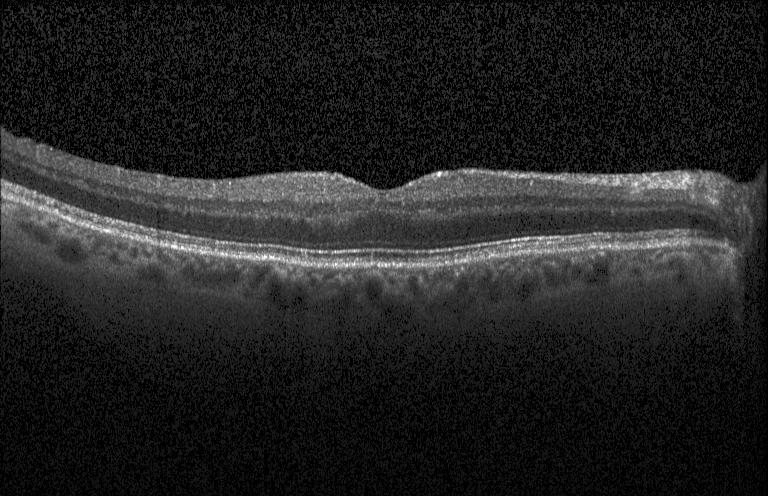 Retinal OCT cross-section, SD-OCT, acquired on a Heidelberg Spectralis, macular scan — Finding: neither choroidal neovascularization, diabetic macular edema, nor drusen.